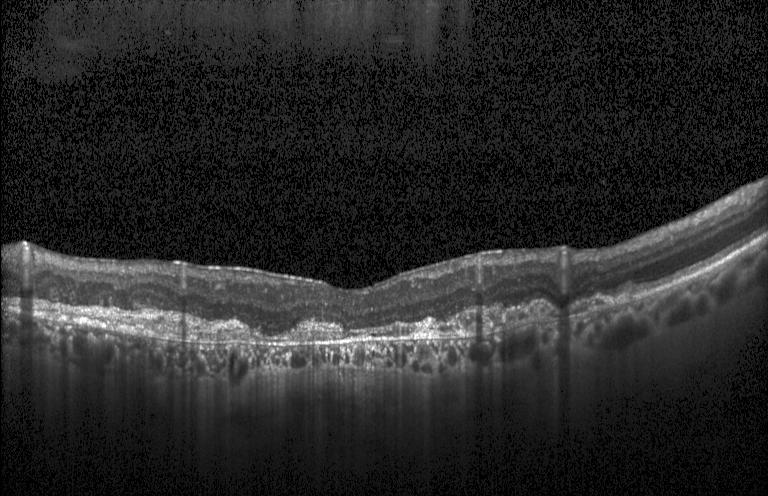

OCT B-scan showing CNV.